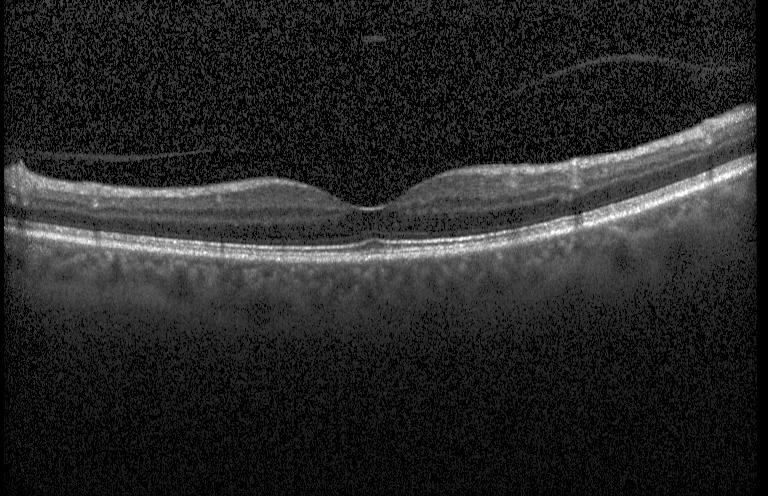
Diagnosis: no CNV, no DME, and no drusen.